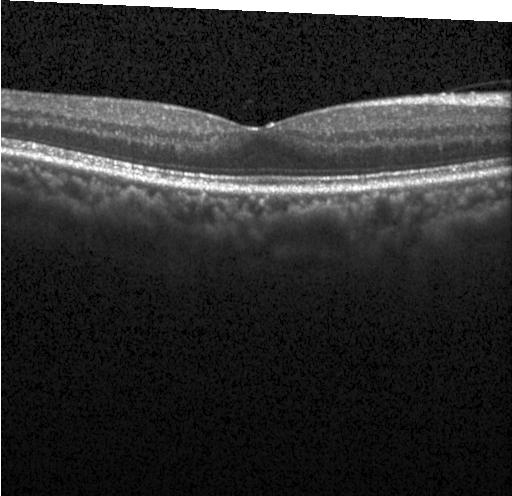 Optical coherence tomography B-scan · Heidelberg Spectralis — Finding: no evidence of choroidal neovascularization, diabetic macular edema, or drusen.